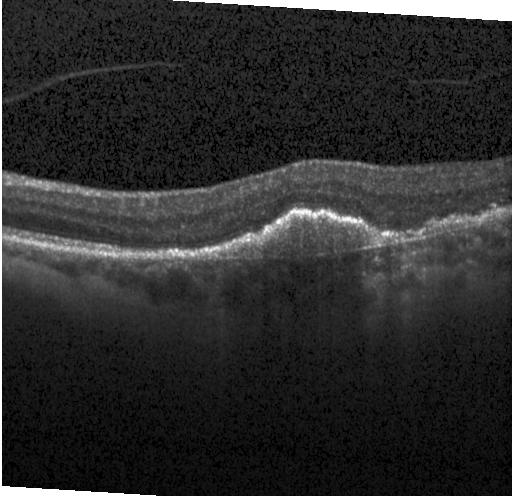 Heidelberg Spectralis OCT system. Retinal OCT cross-section. Horizontal scan through the fovea. SD-OCT
Impression: a choroidal neovascular membrane.